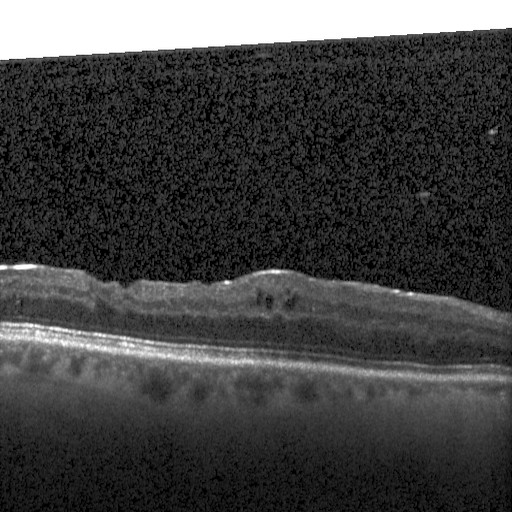

OCT line scan — This B-scan demonstrates DME.